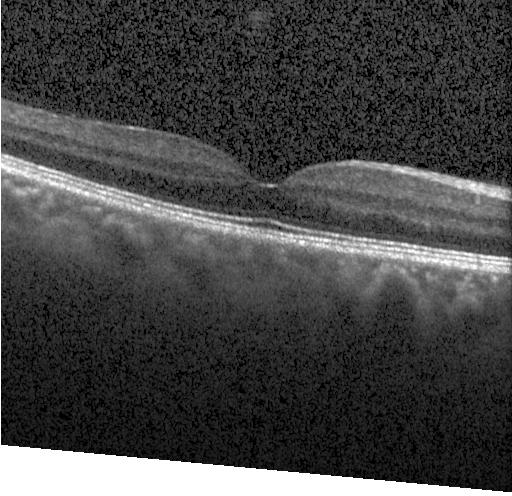 Neither CNV, DME, nor drusen.